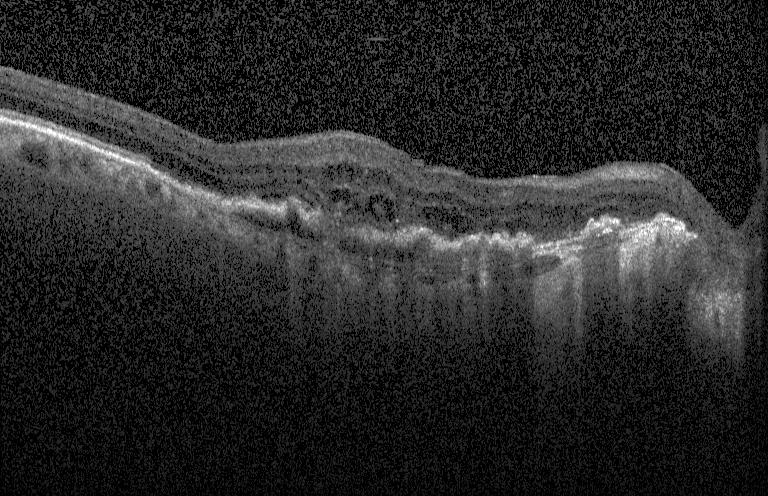

Retinal OCT cross-section — Assessment: a choroidal neovascular membrane.